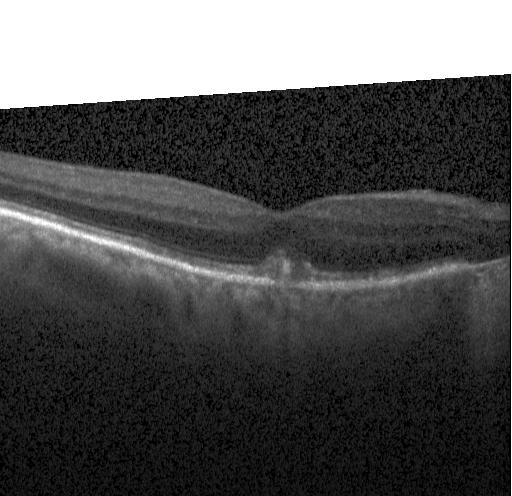

OCT scan showing choroidal neovascularization.